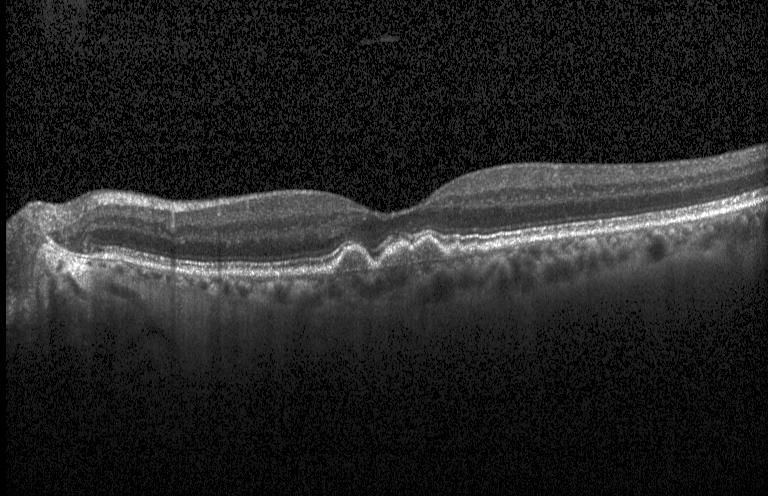
SD-OCT, OCT line scan, Heidelberg Spectralis OCT system — Sub-RPE drusenoid deposits.